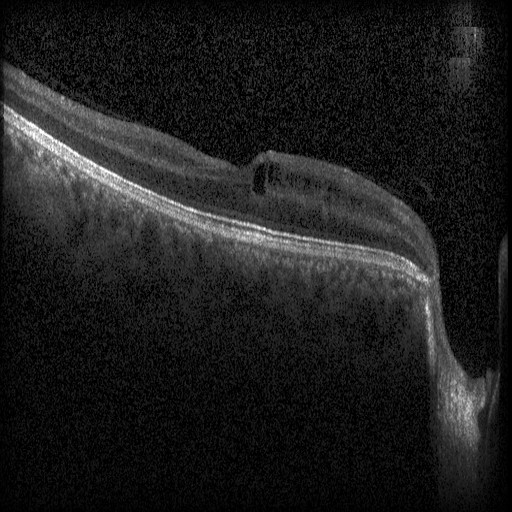
Dx: diabetic macular edema.